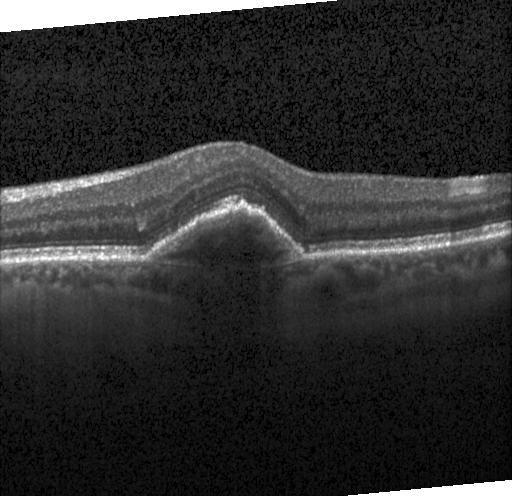

Heidelberg Spectralis OCT system; optical coherence tomography B-scan — The scan shows a choroidal neovascular membrane.